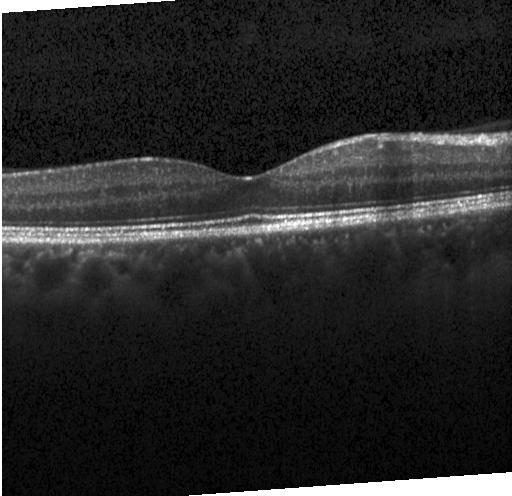
Fovea-centered; optical coherence tomography B-scan; acquired on a Heidelberg Spectralis; spectral-domain optical coherence tomography.
Diagnosis: no evidence of CNV, DME, or drusen.